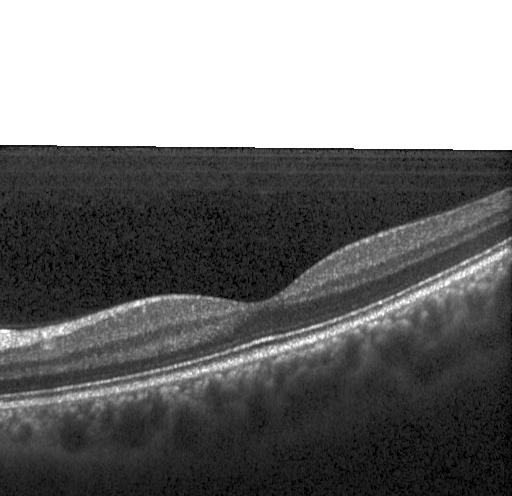 Centered on the fovea. OCT line scan
Finding: no choroidal neovascularization, no diabetic macular edema, and no drusen.